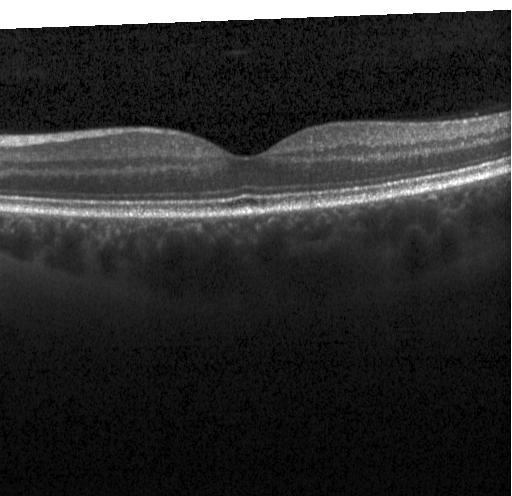
Spectral-domain OCT. Retinal OCT cross-section. Centered on the fovea. Heidelberg Spectralis OCT system. This B-scan demonstrates no choroidal neovascularization, no diabetic macular edema, and no drusen.